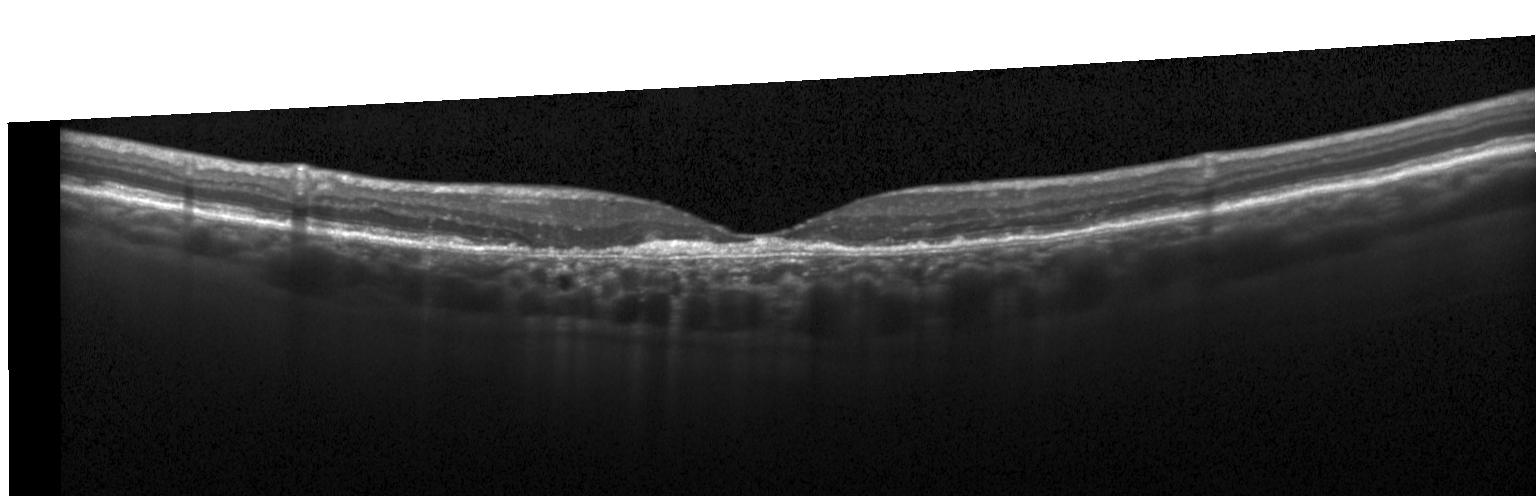 Retinal OCT cross-section.
Finding: a choroidal neovascular membrane.